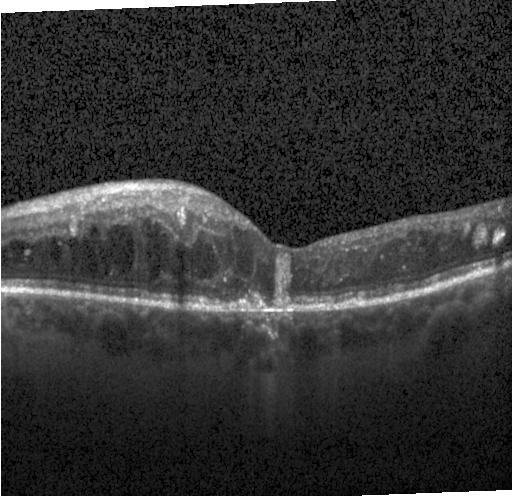
Spectral-domain optical coherence tomography, OCT line scan, fovea-centered, Heidelberg Spectralis OCT system — Macular OCT: DME.